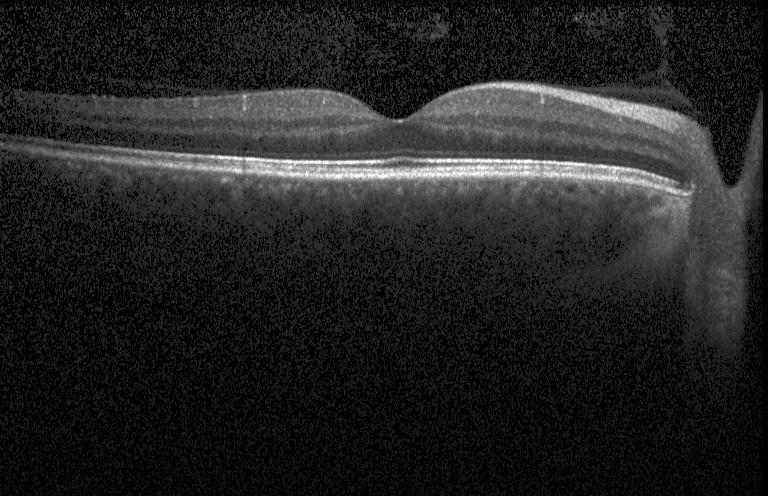
Centered on the fovea; OCT B-scan
This B-scan demonstrates no choroidal neovascularization, no diabetic macular edema, and no drusen.